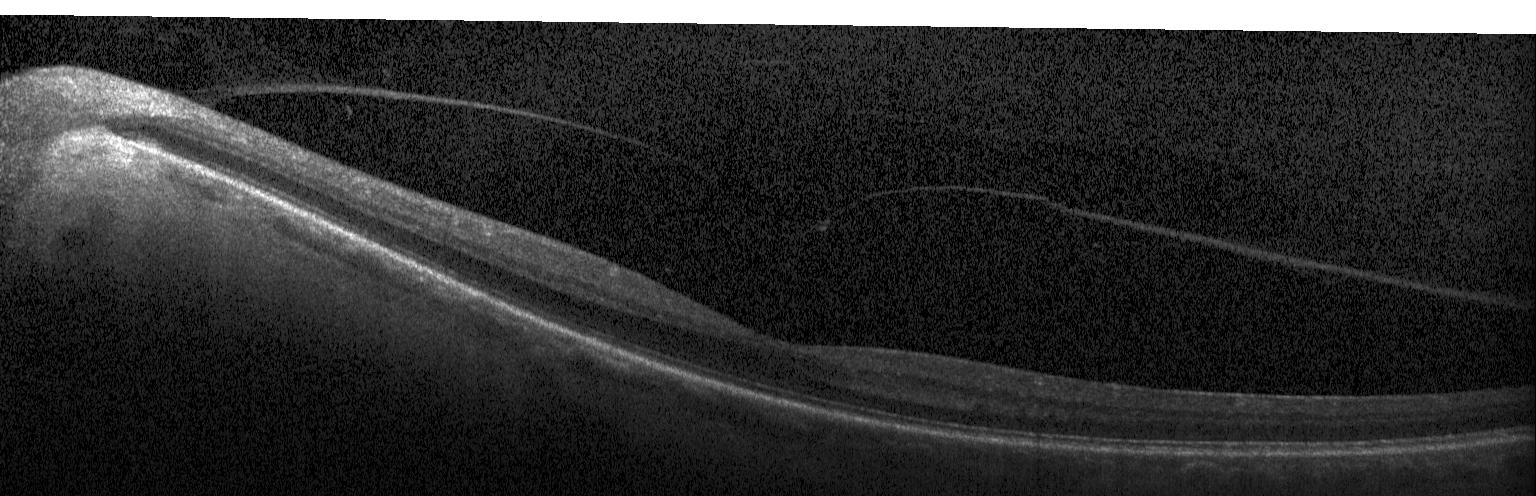
Macular OCT demonstrating neither CNV, DME, nor drusen.